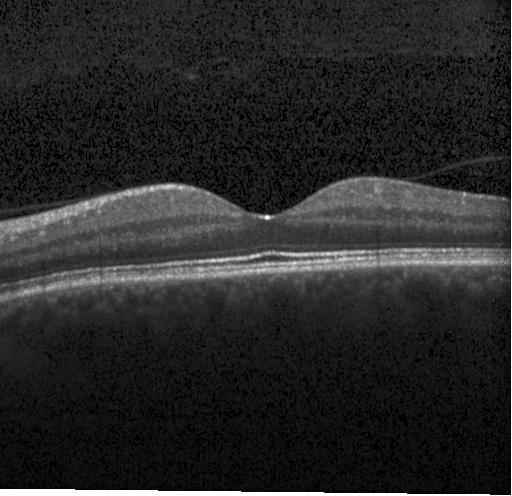
OCT scan showing no CNV, DME, or drusen.